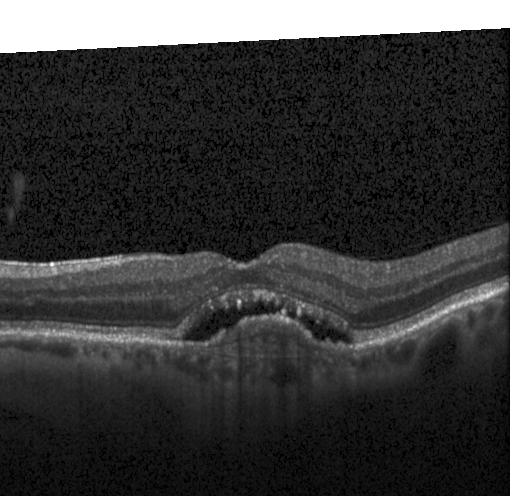
Macular OCT demonstrating choroidal neovascularization.